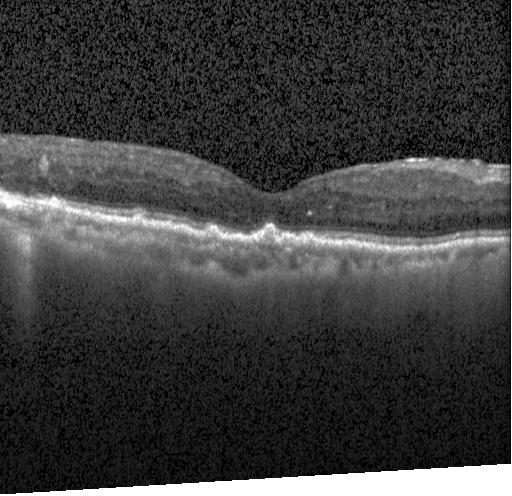
Macular scan · retinal OCT B-scan · spectral-domain optical coherence tomography · instrument: Heidelberg Spectralis — Sub-RPE drusenoid deposits.